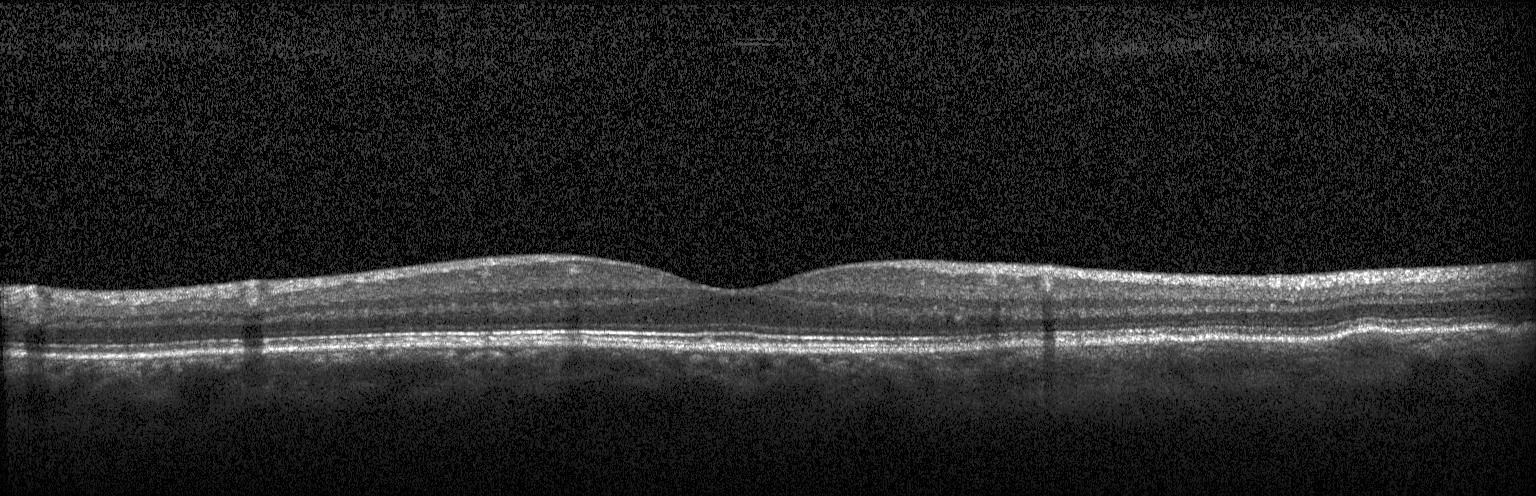 OCT B-scan
Impression: neither CNV, DME, nor drusen.